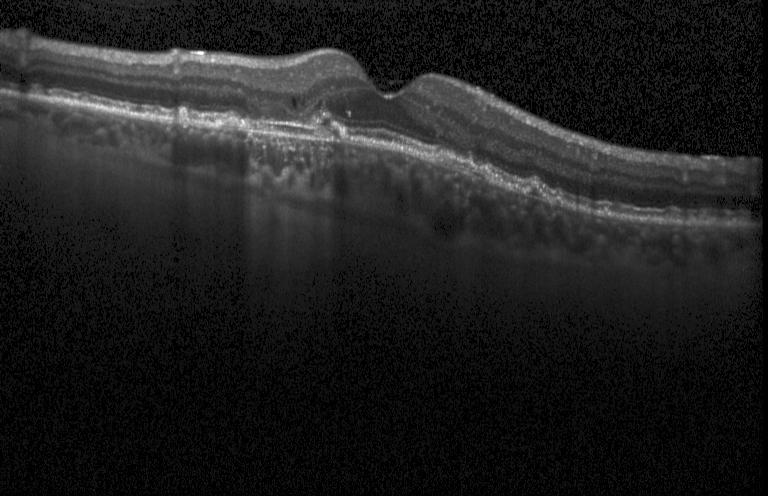

Macular OCT: choroidal neovascularization (CNV).